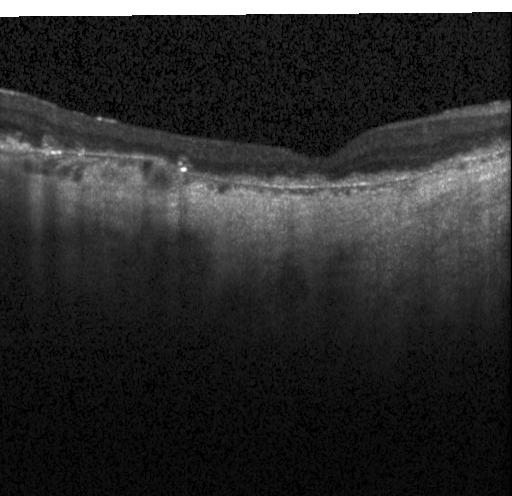 Spectral-domain OCT B-scan: choroidal neovascularization (CNV).